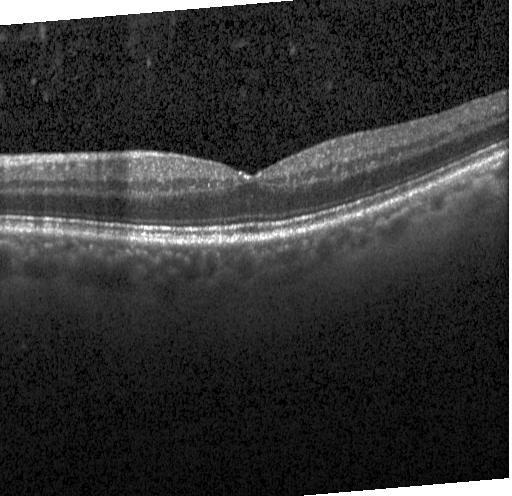

This B-scan demonstrates no evidence of choroidal neovascularization, diabetic macular edema, or drusen.